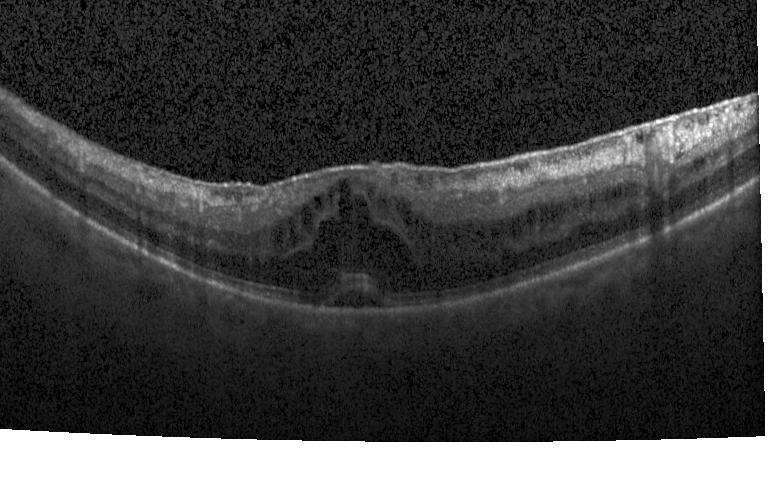

Retinal OCT B-scan · spectral-domain optical coherence tomography — DME.